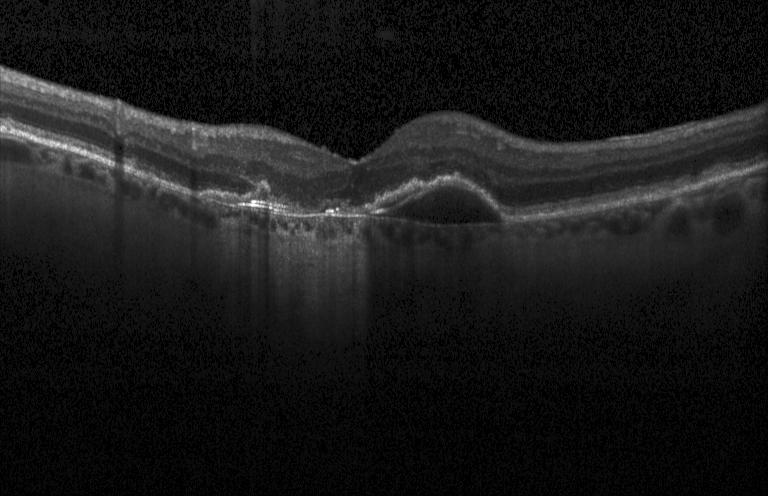 SD-OCT. Optical coherence tomography B-scan
Choroidal neovascularization.